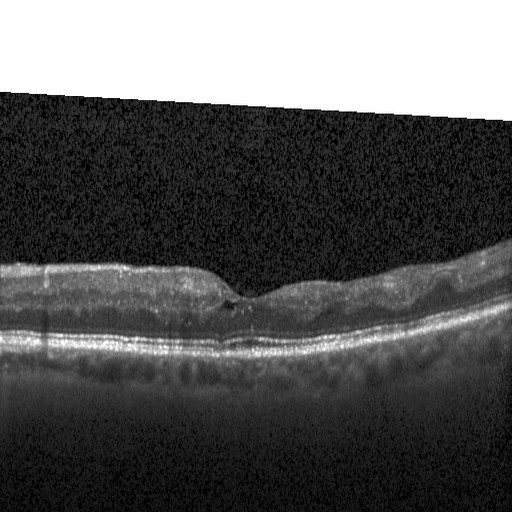

OCT finding: DME.